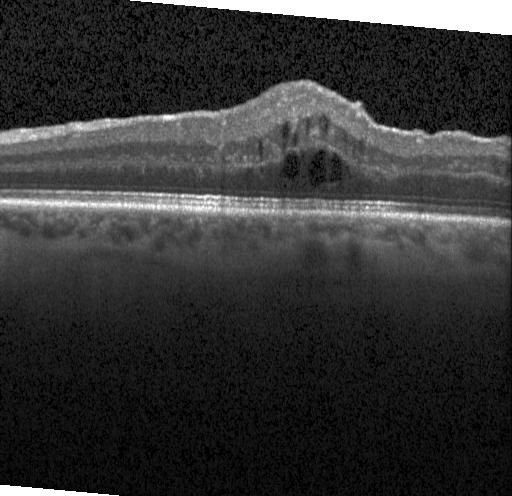
Spectral-domain OCT. Instrument: Heidelberg Spectralis. Retinal OCT B-scan. Through the macula. The scan shows diabetic macular edema.